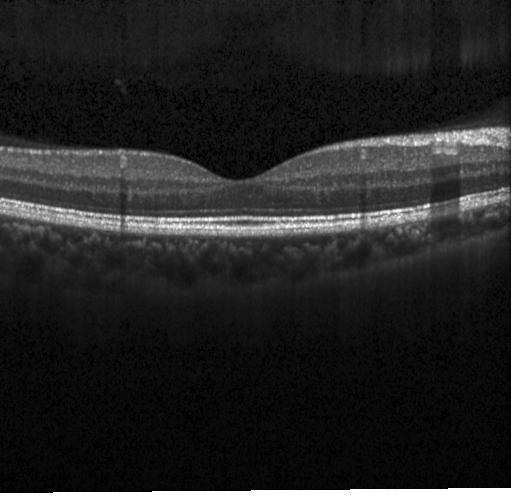

Spectral-domain OCT B-scan: no CNV, no DME, and no drusen.